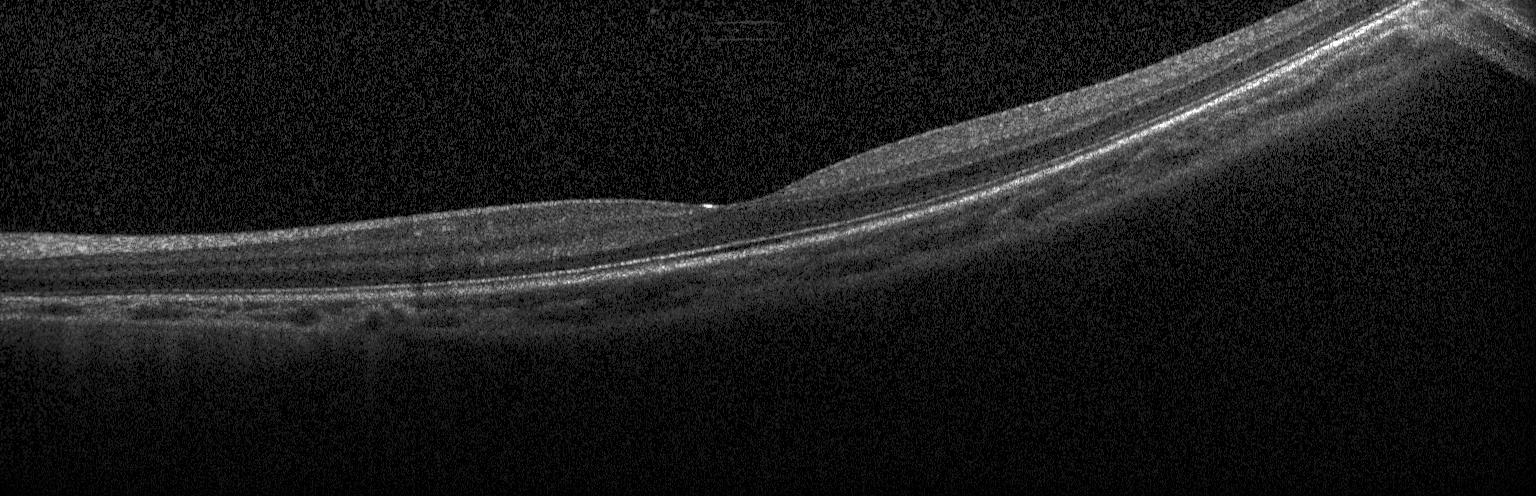
Optical coherence tomography B-scan; centered on the fovea — The scan shows neither choroidal neovascularization, diabetic macular edema, nor drusen.